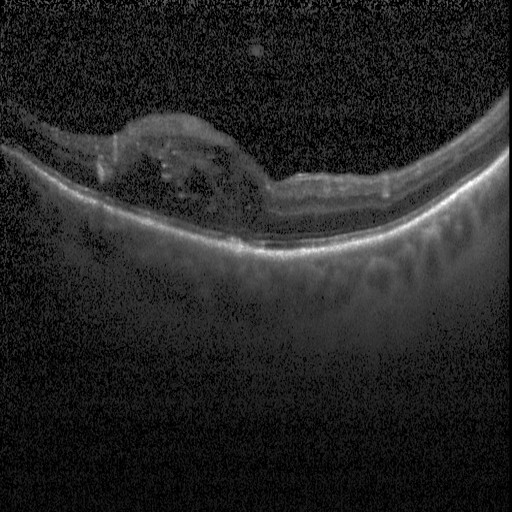 The scan shows diabetic macular edema (DME).